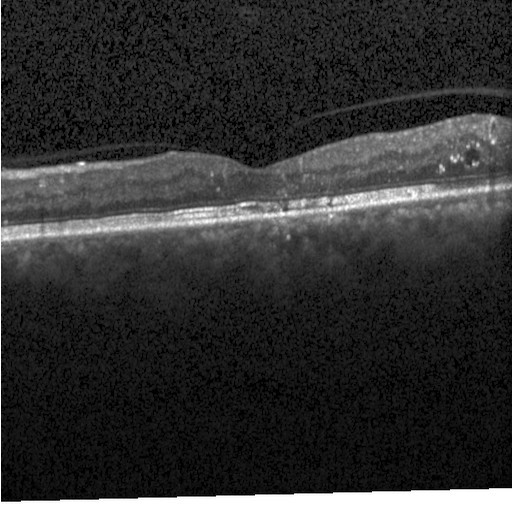

Retinal OCT B-scan — Finding: DME.